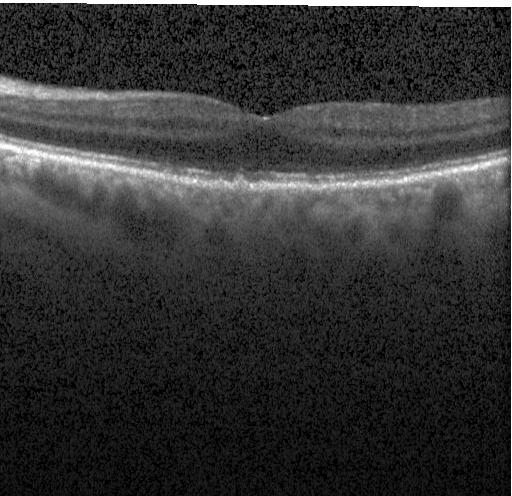 Heidelberg Spectralis OCT system. Retinal OCT B-scan. Fovea-centered
OCT finding: sub-RPE drusenoid deposits.